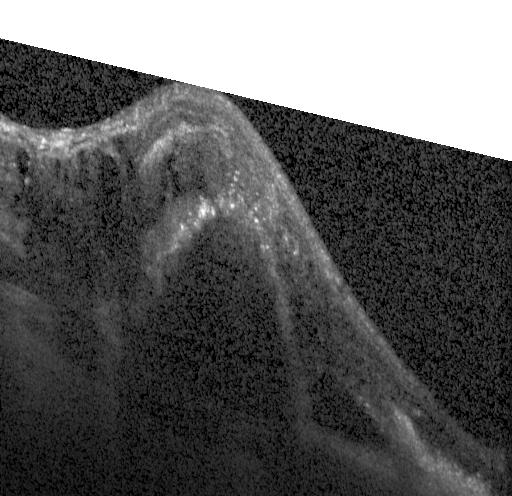 Impression: a choroidal neovascular membrane.